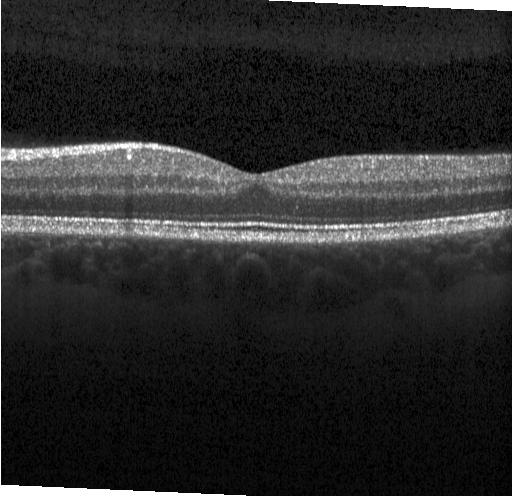 OCT B-scan · spectral-domain OCT — Assessment: no choroidal neovascularization, no diabetic macular edema, and no drusen.